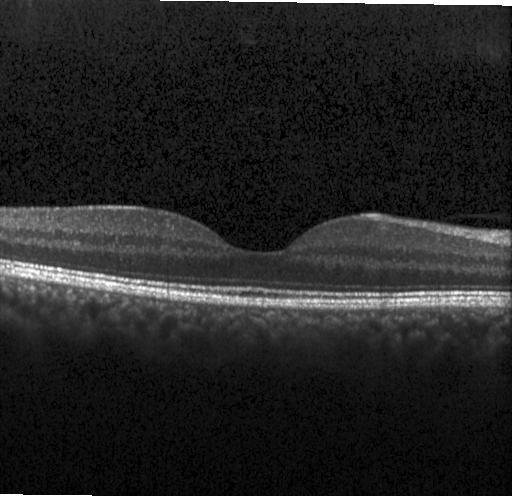 Spectral-domain optical coherence tomography, OCT B-scan. Impression: no CNV, DME, or drusen.